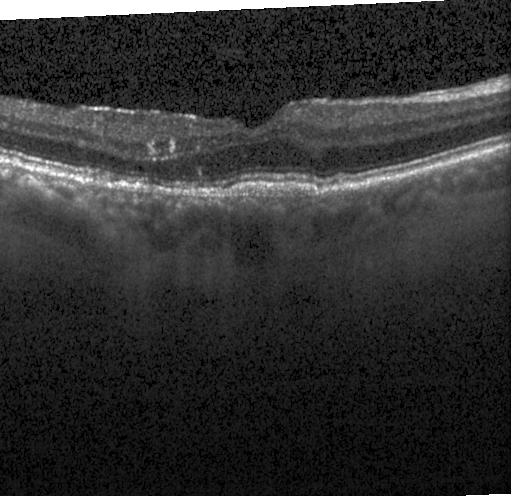

Retinal OCT cross-section showing a choroidal neovascular membrane.